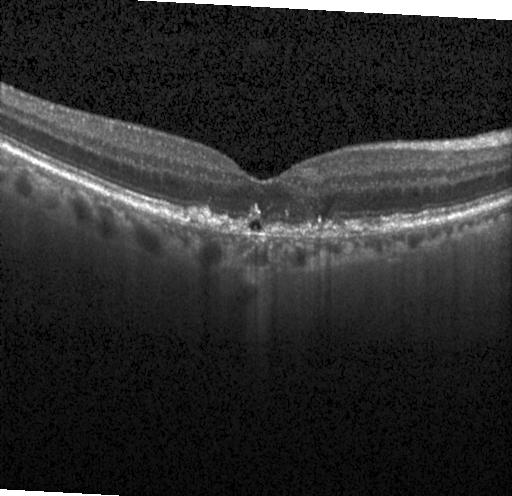 OCT line scan · Heidelberg Spectralis — This B-scan demonstrates a choroidal neovascular membrane.